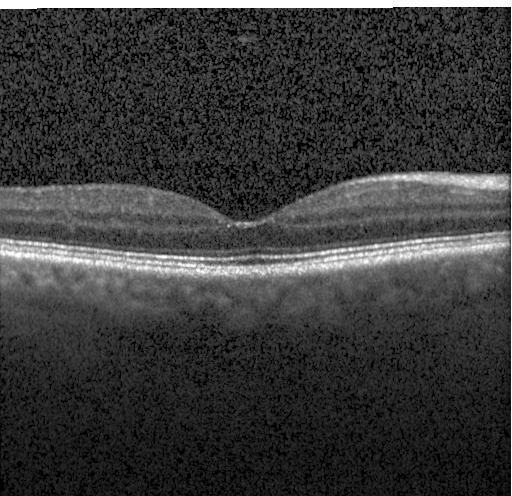
Spectral-domain OCT · OCT B-scan · Heidelberg Spectralis OCT system · centered on the fovea. OCT finding: no choroidal neovascularization, diabetic macular edema, or drusen.